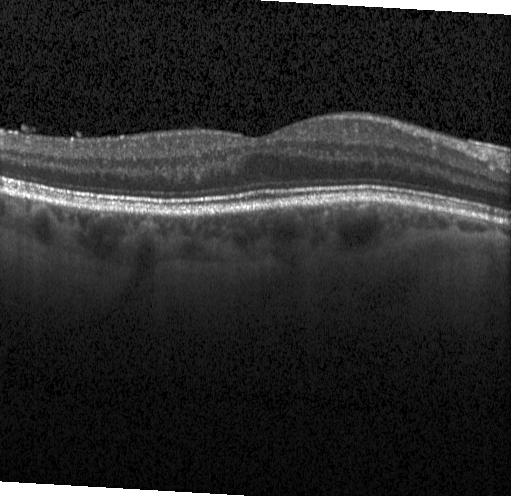
Centered on the fovea; OCT B-scan; spectral-domain optical coherence tomography; acquired on a Heidelberg Spectralis — Impression: neither choroidal neovascularization, diabetic macular edema, nor drusen.